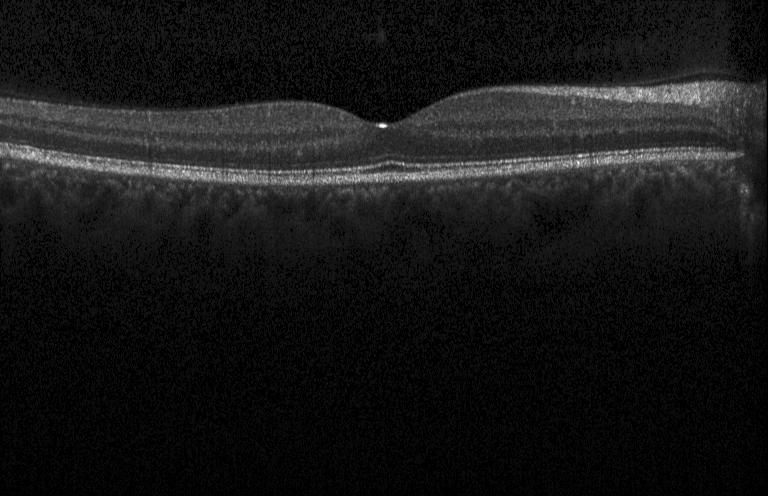 OCT finding: no CNV, no DME, and no drusen.